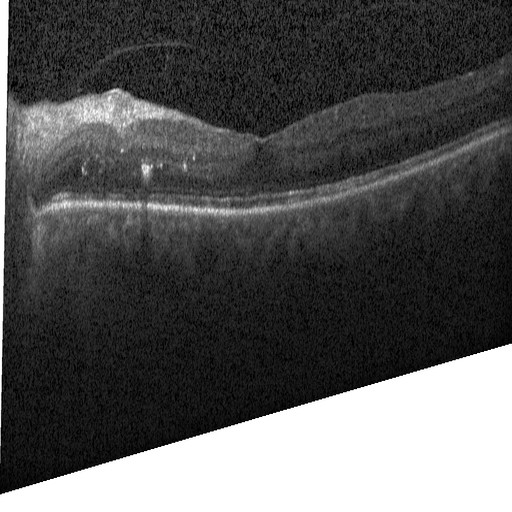

Impression: diabetic macular edema (DME).